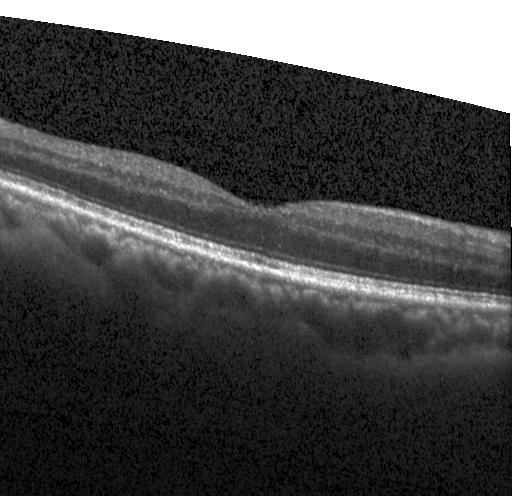

The scan shows no evidence of choroidal neovascularization, diabetic macular edema, or drusen.